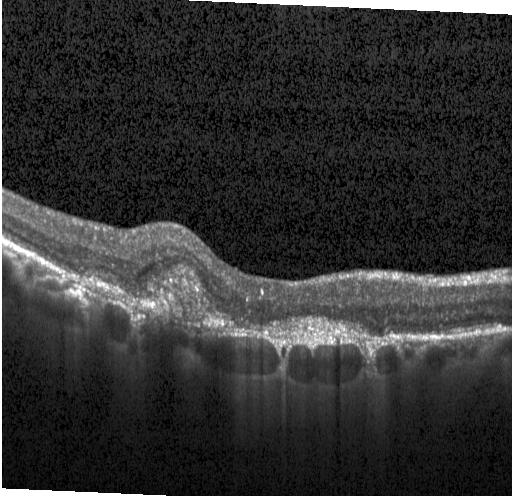

Impression: choroidal neovascularization.